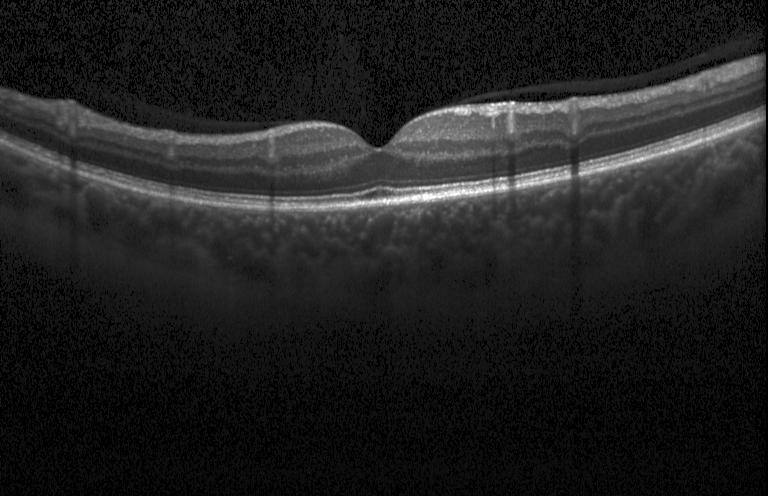 Heidelberg Spectralis · OCT B-scan · SD-OCT. Diagnosis: no choroidal neovascularization, no diabetic macular edema, and no drusen.